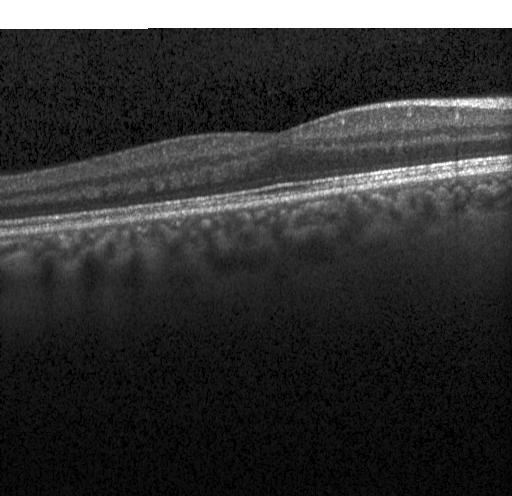
Instrument: Heidelberg Spectralis · optical coherence tomography scan
Assessment: neither choroidal neovascularization, diabetic macular edema, nor drusen.